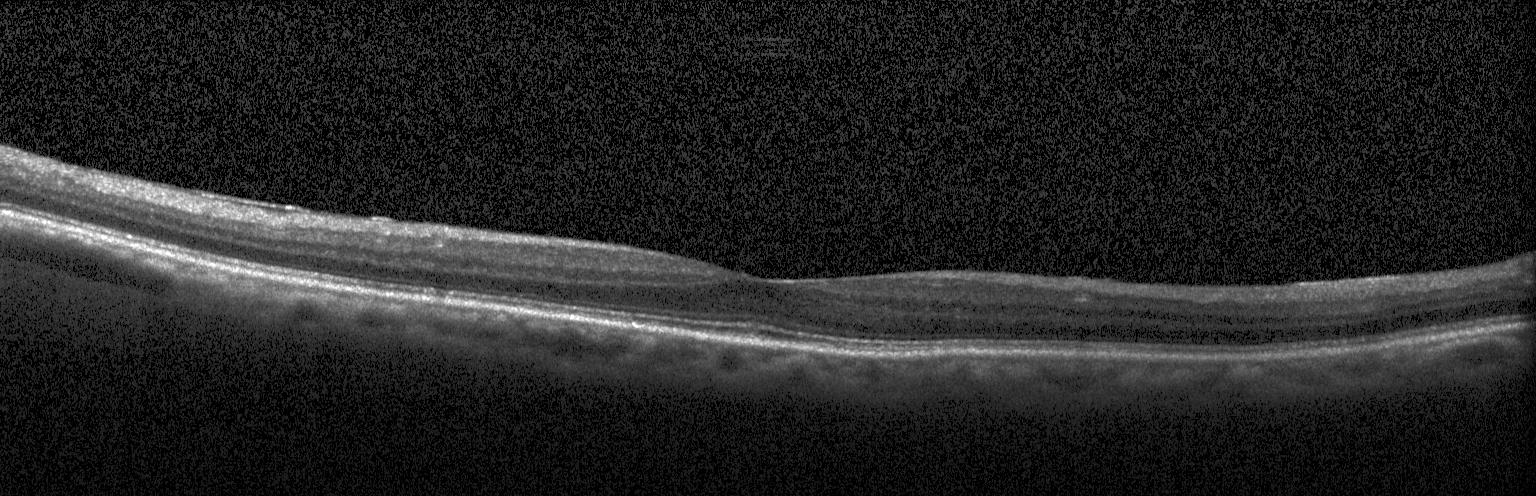

Retinal OCT cross-section; spectral-domain optical coherence tomography.
Assessment: neither choroidal neovascularization, diabetic macular edema, nor drusen.